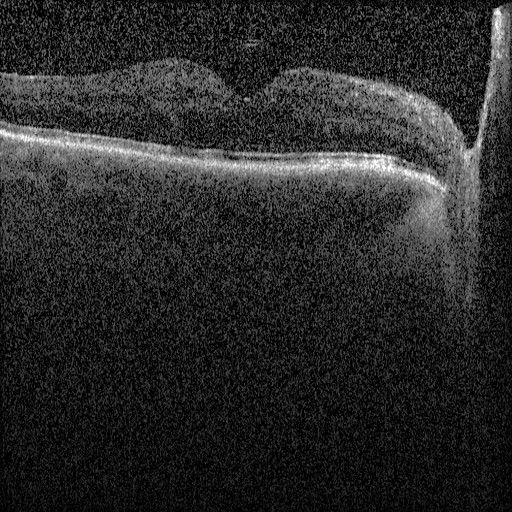 OCT line scan; horizontal scan through the fovea; Heidelberg Spectralis OCT system — Diagnosis: DME.